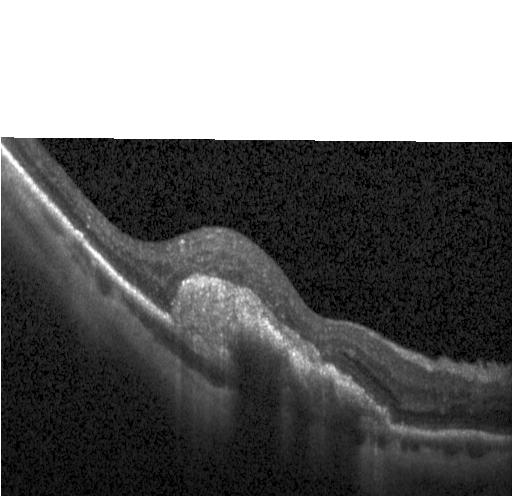 Macular OCT: a choroidal neovascular membrane.